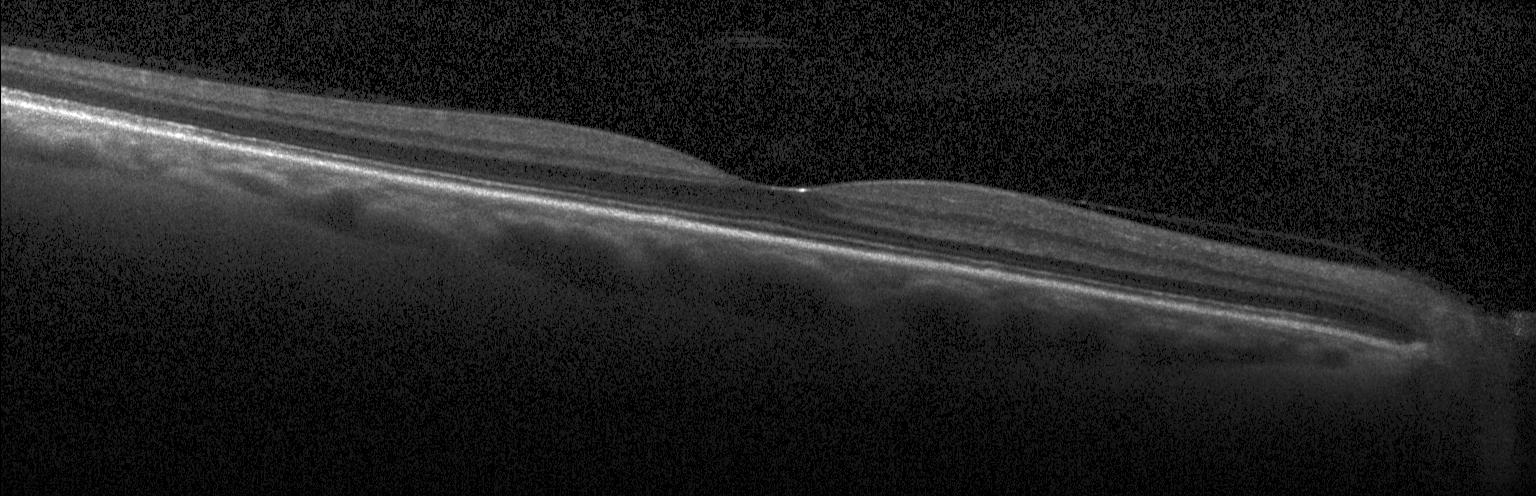
OCT finding: neither CNV, DME, nor drusen.